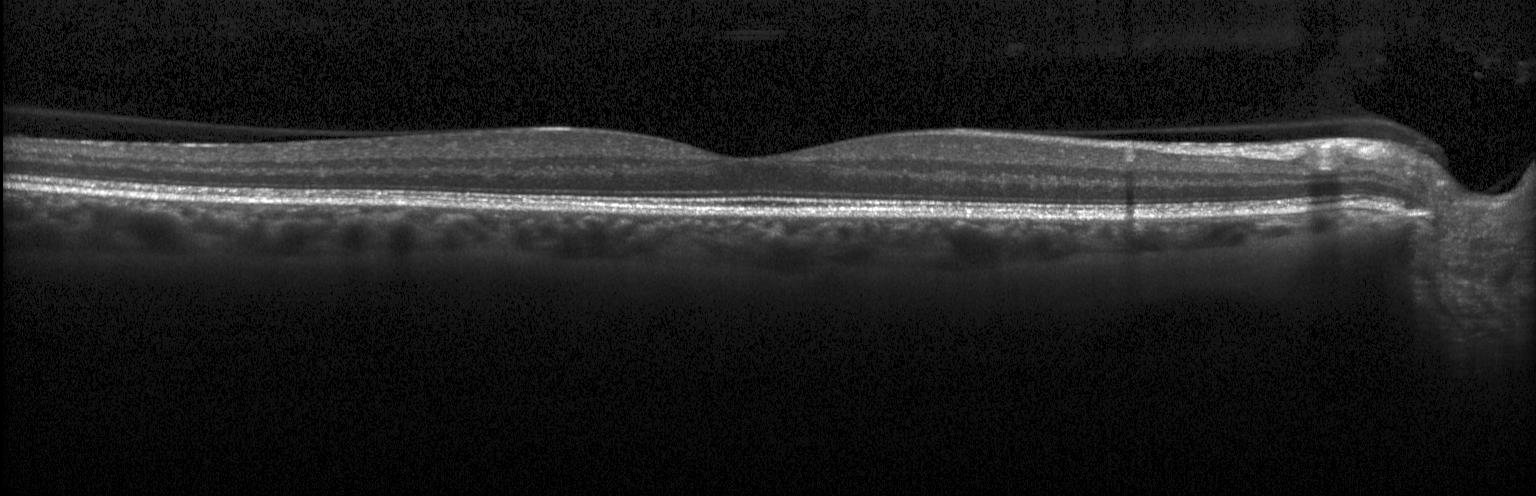
OCT line scan
The scan shows no CNV, DME, or drusen.